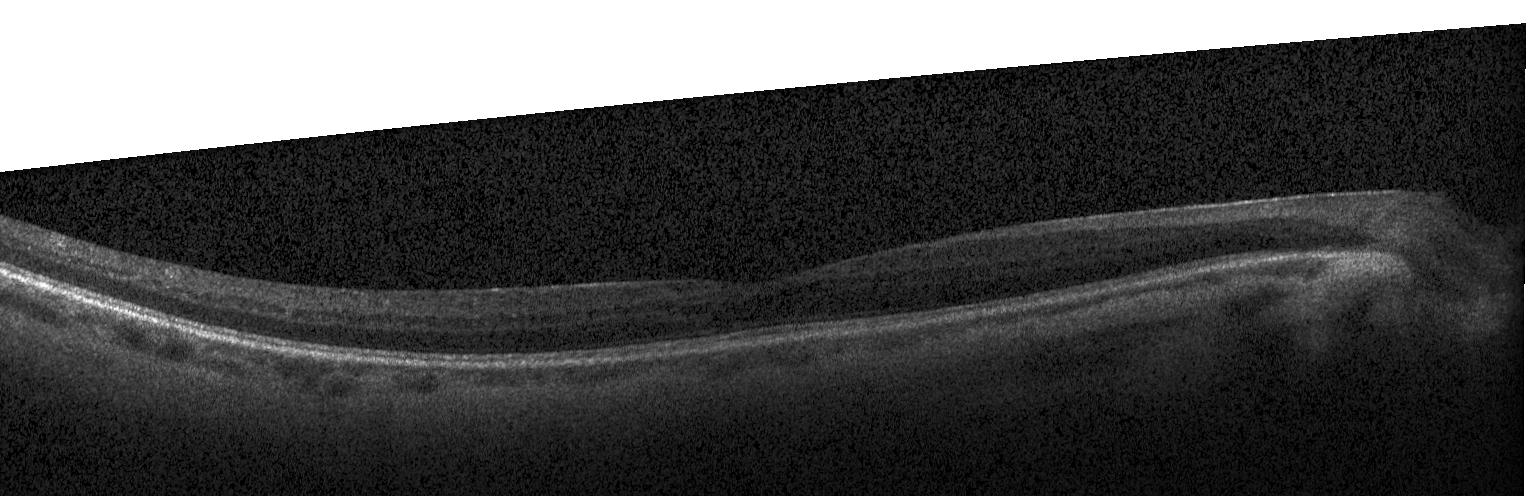

OCT B-scan; spectral-domain optical coherence tomography; instrument: Heidelberg Spectralis; through the macula
Impression: neither CNV, DME, nor drusen.